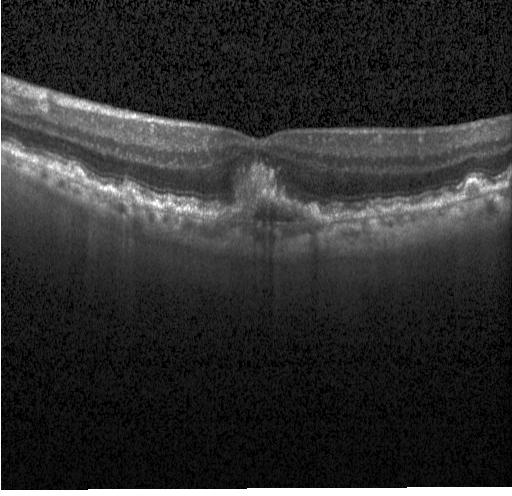
Dx: choroidal neovascularization (CNV).